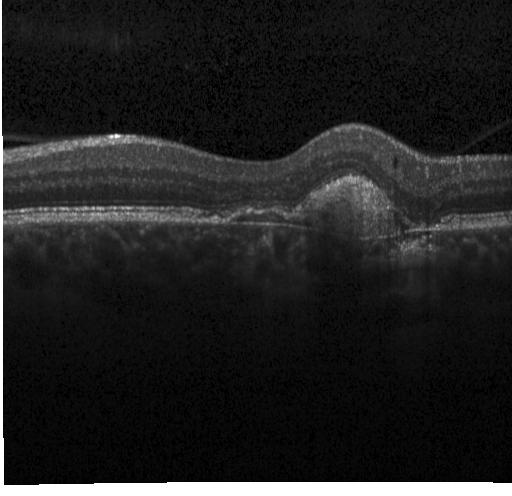
Finding: a choroidal neovascular membrane.